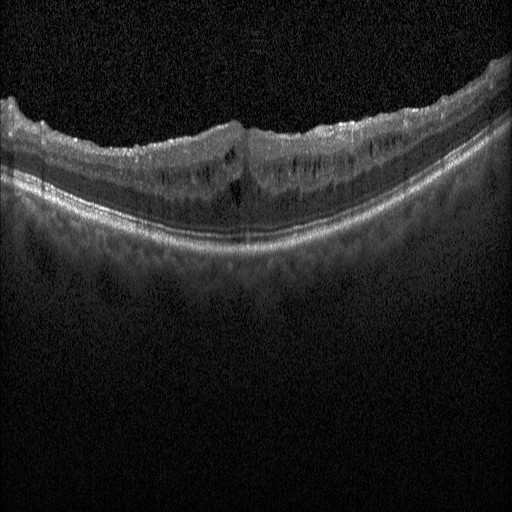 Horizontal scan through the fovea; spectral-domain OCT; retinal OCT B-scan
OCT finding: diabetic macular edema.